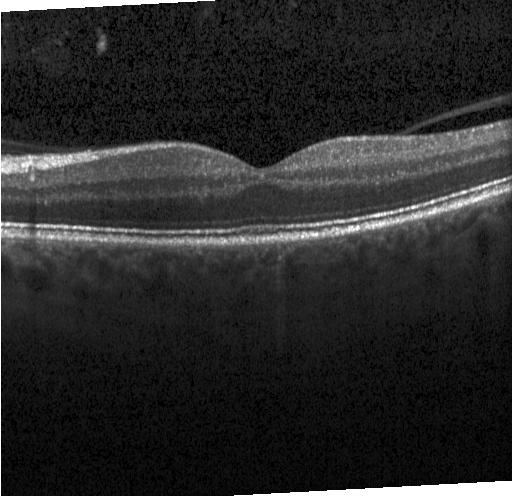
Optical coherence tomography scan. Dx: neither choroidal neovascularization, diabetic macular edema, nor drusen.